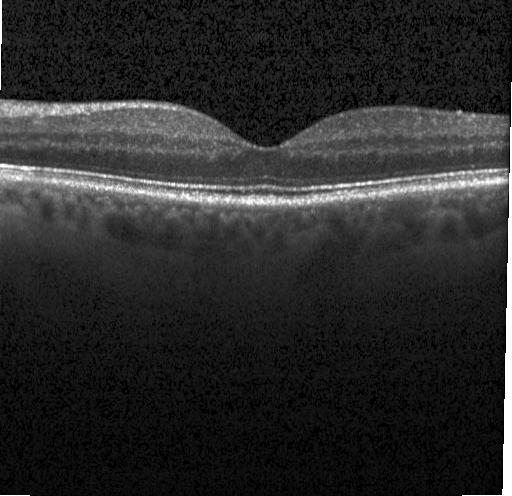 Diagnosis: no evidence of CNV, DME, or drusen.